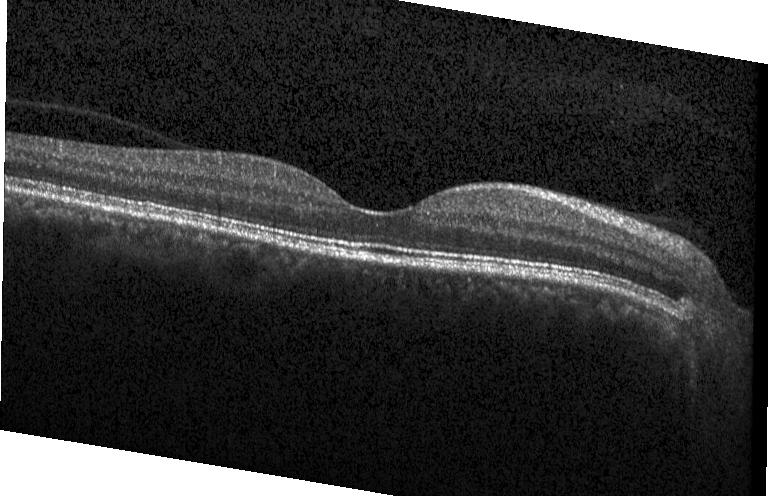

OCT B-scan. Finding: neither choroidal neovascularization, diabetic macular edema, nor drusen.